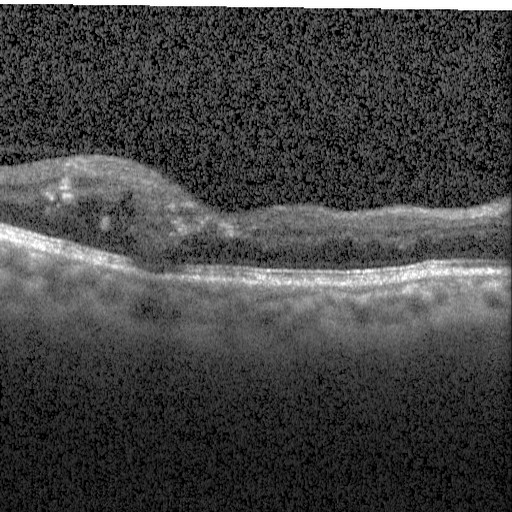

Heidelberg Spectralis OCT system, retinal OCT B-scan — DME.